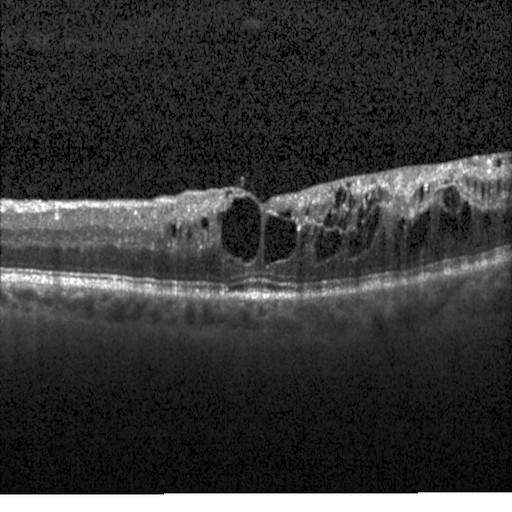
SD-OCT; through the macula; Heidelberg Spectralis OCT system; OCT B-scan — Assessment: DME.